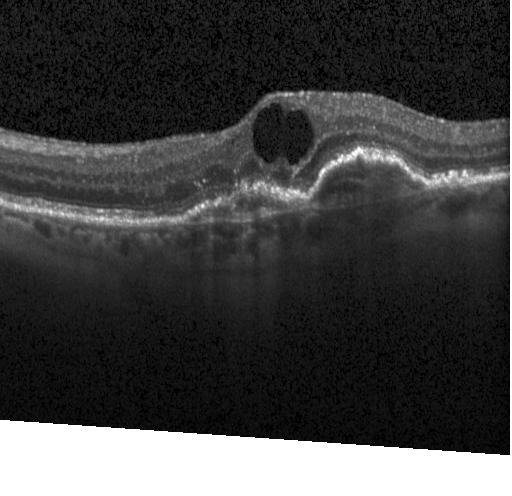
The scan shows a choroidal neovascular membrane.